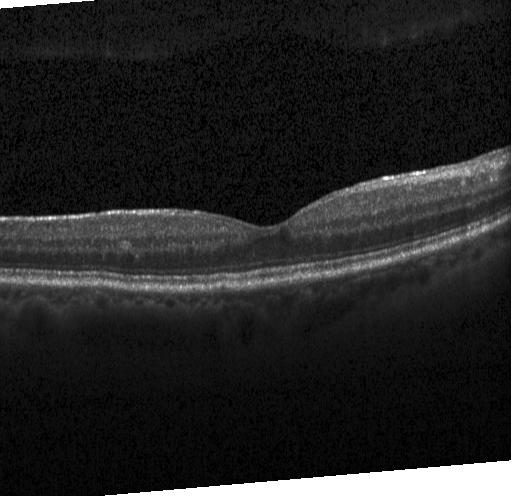 Macular OCT demonstrating no evidence of choroidal neovascularization, diabetic macular edema, or drusen.